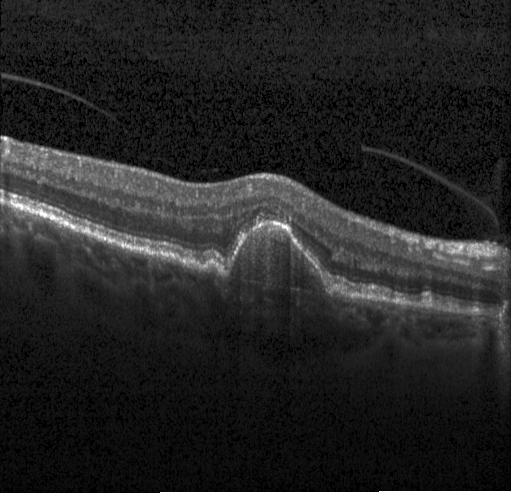 Optical coherence tomography scan · instrument: Heidelberg Spectralis · centered on the fovea.
Assessment: choroidal neovascularization.